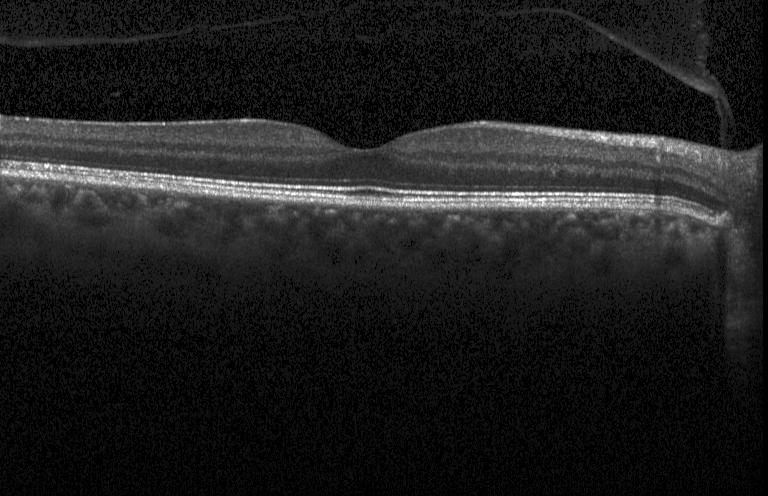
OCT B-scan showing neither choroidal neovascularization, diabetic macular edema, nor drusen.